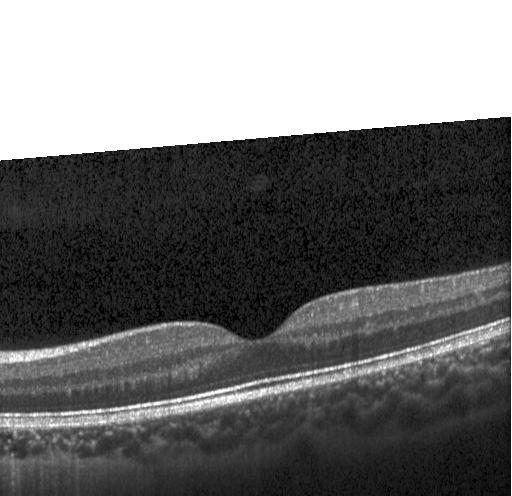

Impression: no evidence of CNV, DME, or drusen.